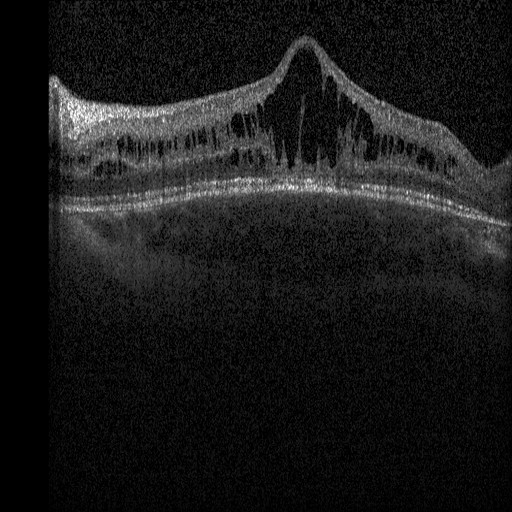

OCT finding: diabetic macular edema.